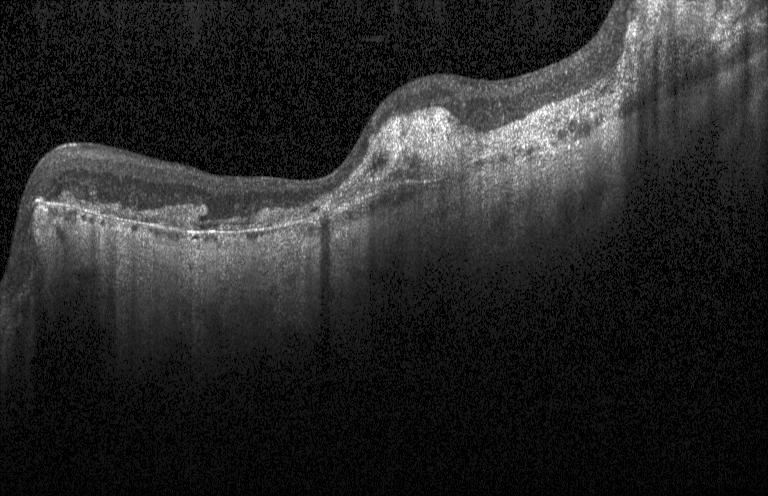
Through the macula, optical coherence tomography scan.
Impression: a choroidal neovascular membrane.